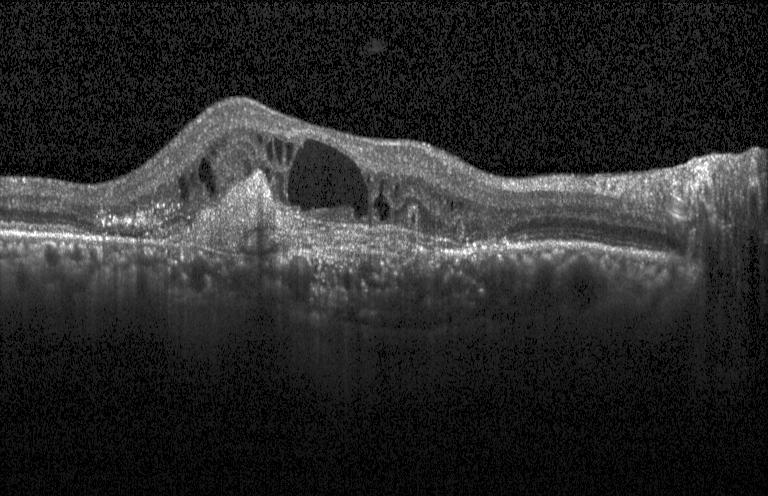 OCT B-scan showing choroidal neovascularization.